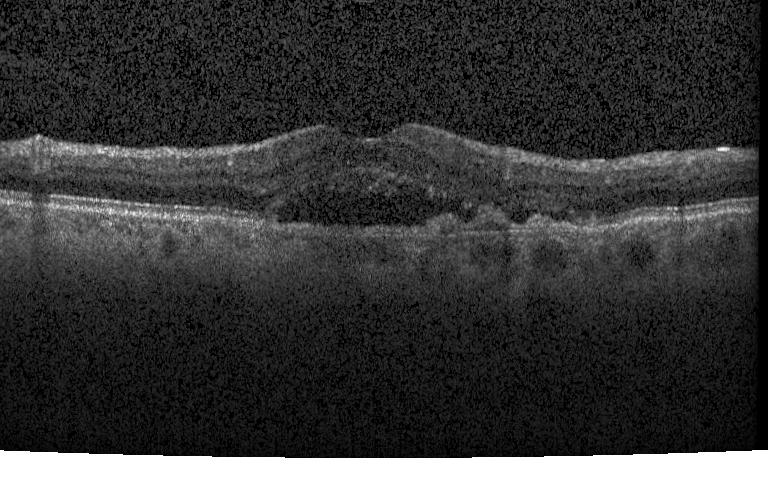

SD-OCT; through the macula; optical coherence tomography B-scan; Heidelberg Spectralis.
The scan shows a choroidal neovascular membrane.